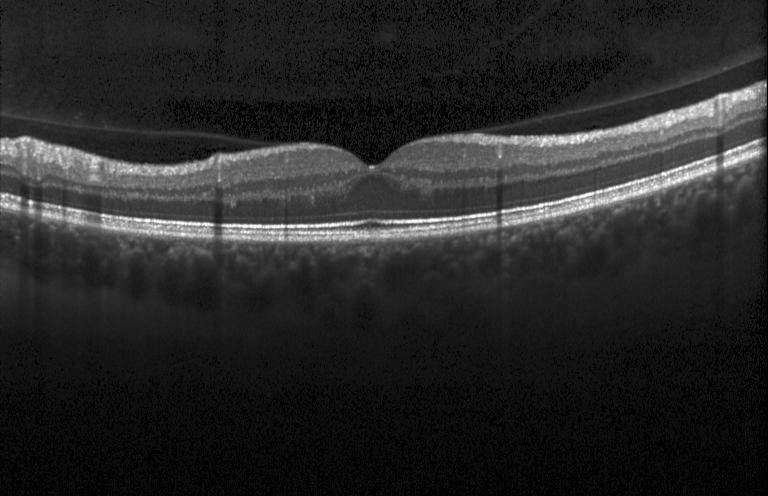

Retinal OCT cross-section.
Impression: no choroidal neovascularization, diabetic macular edema, or drusen.